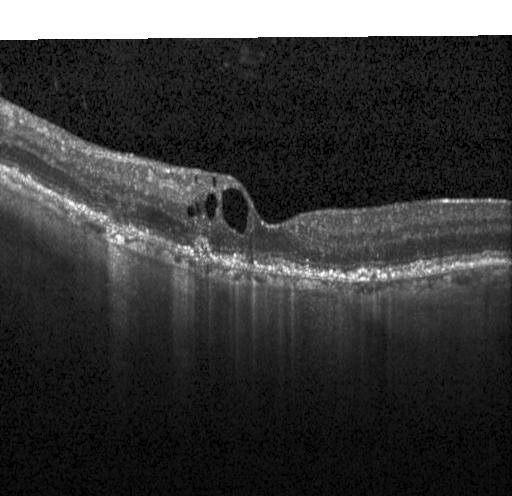
Fovea-centered. SD-OCT. Retinal OCT B-scan. Acquired on a Heidelberg Spectralis.
Finding: a choroidal neovascular membrane.